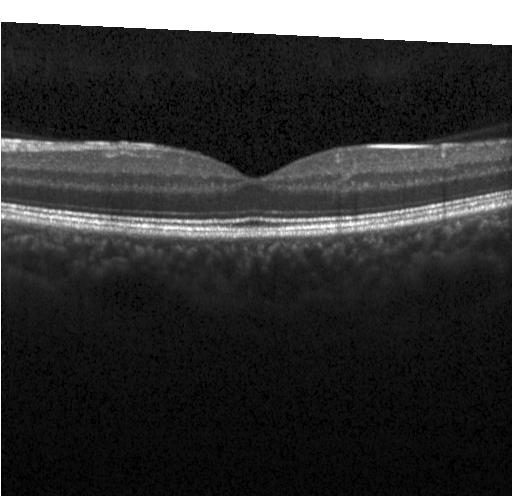 Through the macula; Heidelberg Spectralis; optical coherence tomography B-scan — The scan shows neither choroidal neovascularization, diabetic macular edema, nor drusen.